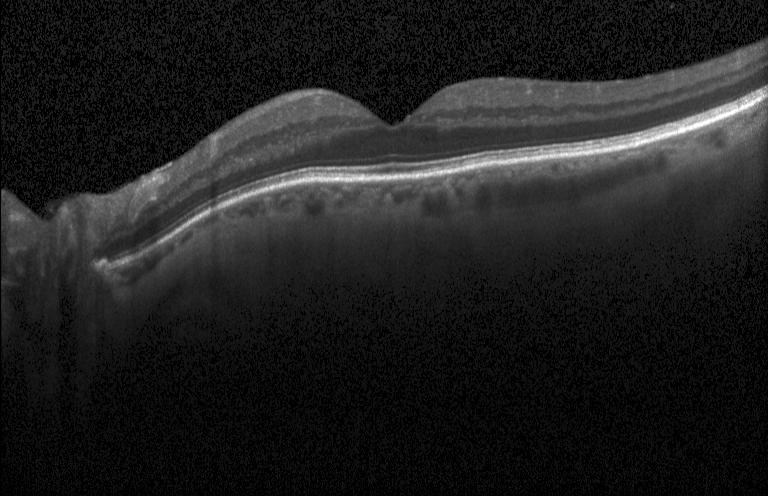
This B-scan demonstrates neither choroidal neovascularization, diabetic macular edema, nor drusen.